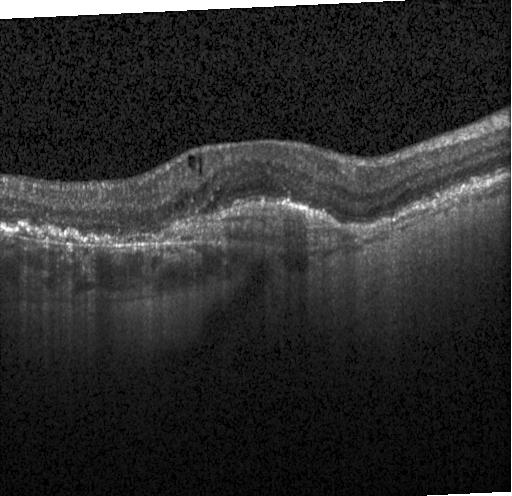

Through the macula; OCT B-scan — Finding: a choroidal neovascular membrane.